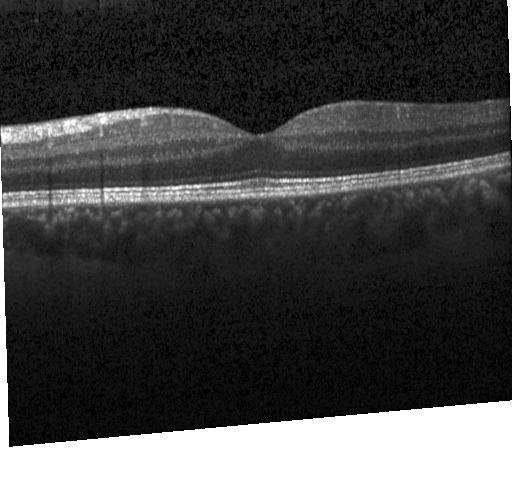

Heidelberg Spectralis · retinal OCT cross-section.
This B-scan demonstrates neither CNV, DME, nor drusen.